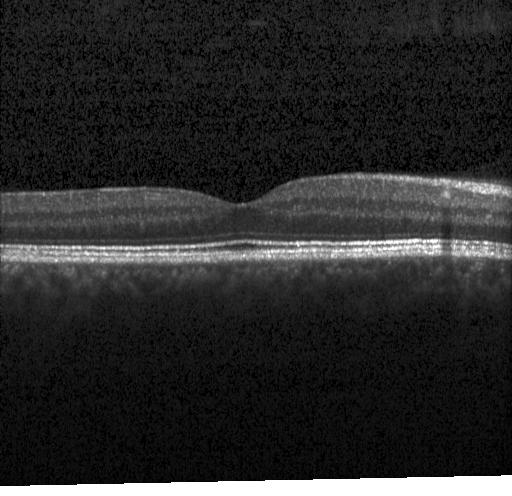
Retinal OCT cross-section, spectral-domain OCT, Heidelberg Spectralis OCT system.
Finding: no choroidal neovascularization, no diabetic macular edema, and no drusen.